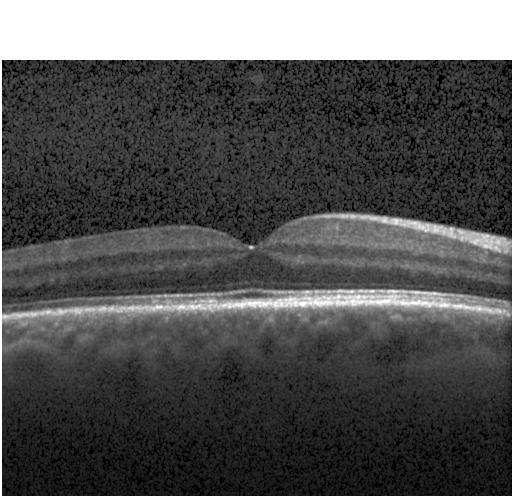
Spectral-domain OCT B-scan: no evidence of CNV, DME, or drusen.